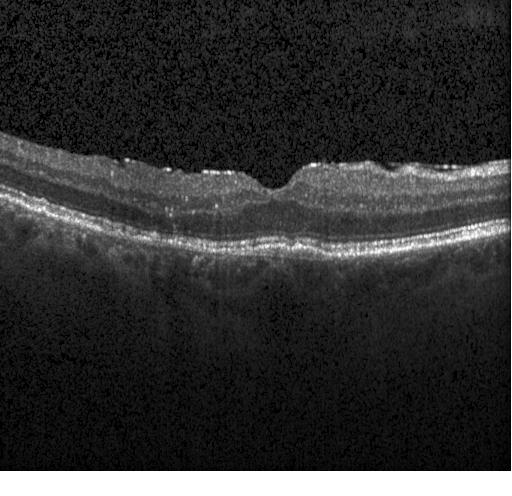 Retinal OCT cross-section, horizontal scan through the fovea, acquired on a Heidelberg Spectralis, spectral-domain optical coherence tomography
Diagnosis: choroidal neovascularization (CNV).